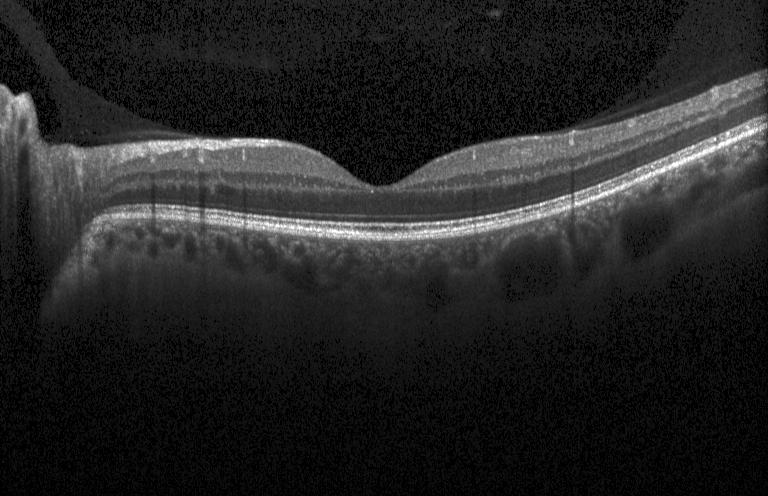
Retinal OCT cross-section. Acquired on a Heidelberg Spectralis. Assessment: no CNV, DME, or drusen.